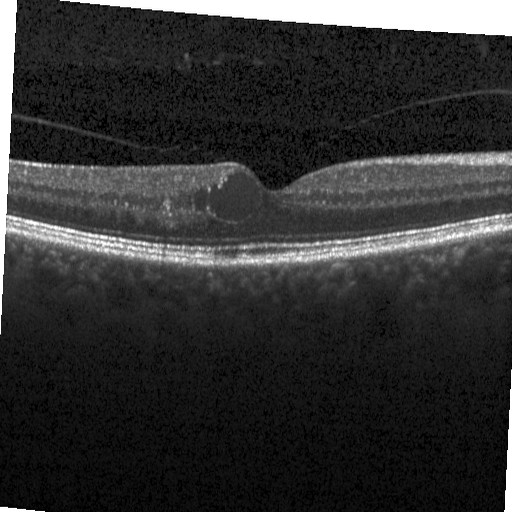
Finding: diabetic macular edema (DME).